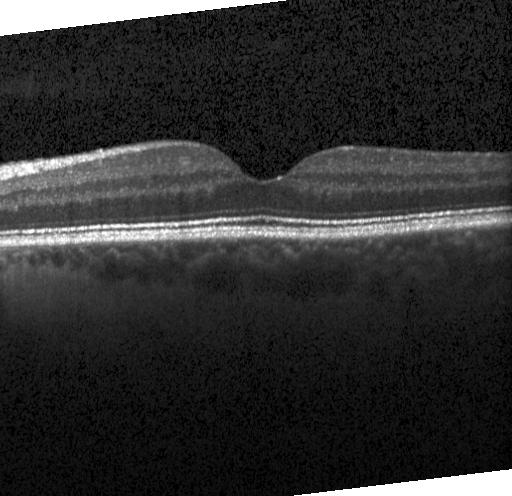

OCT B-scan. Centered on the fovea. Instrument: Heidelberg Spectralis. OCT finding: no CNV, DME, or drusen.